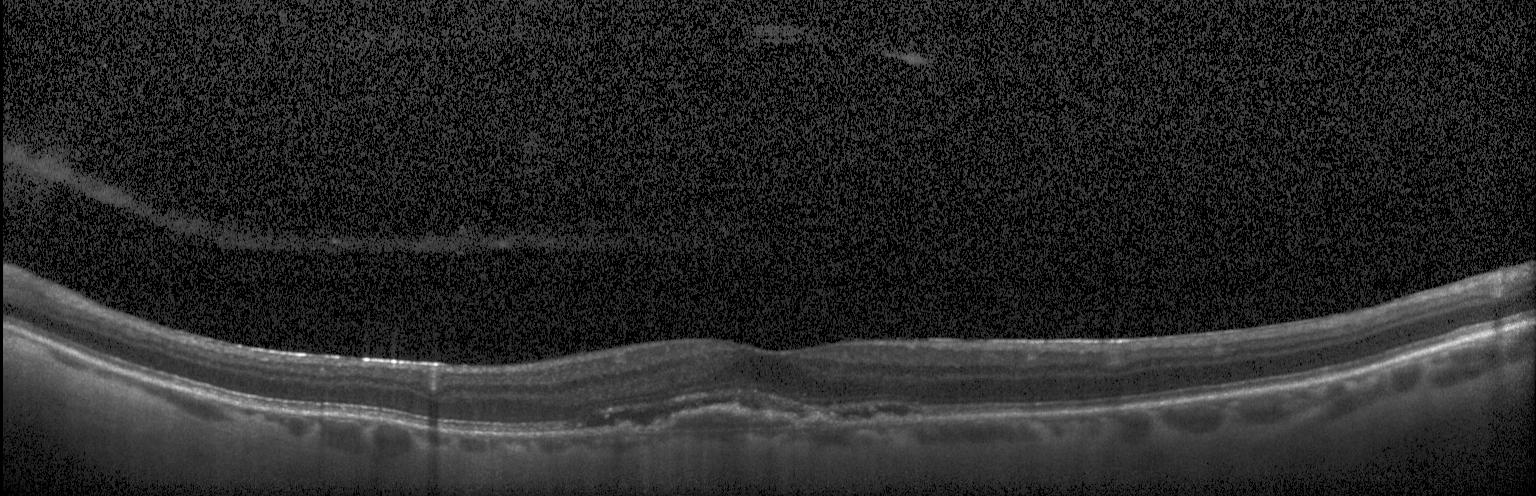

Spectral-domain OCT; retinal OCT B-scan; acquired on a Heidelberg Spectralis; macular scan
Diagnosis: a choroidal neovascular membrane.